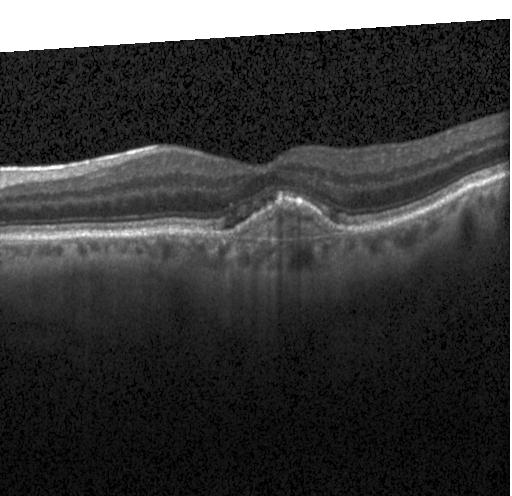
Macular OCT: a choroidal neovascular membrane.